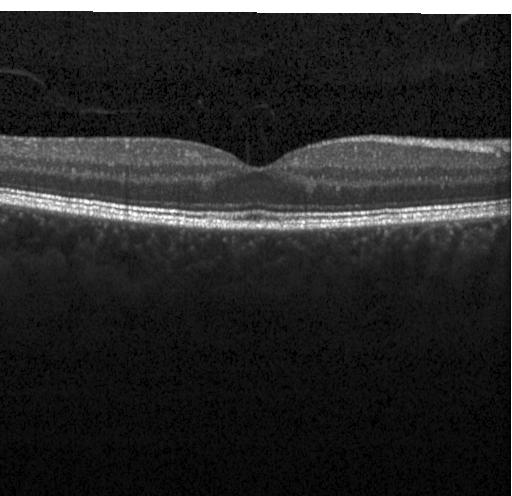
OCT B-scan.
Finding: no choroidal neovascularization, no diabetic macular edema, and no drusen.